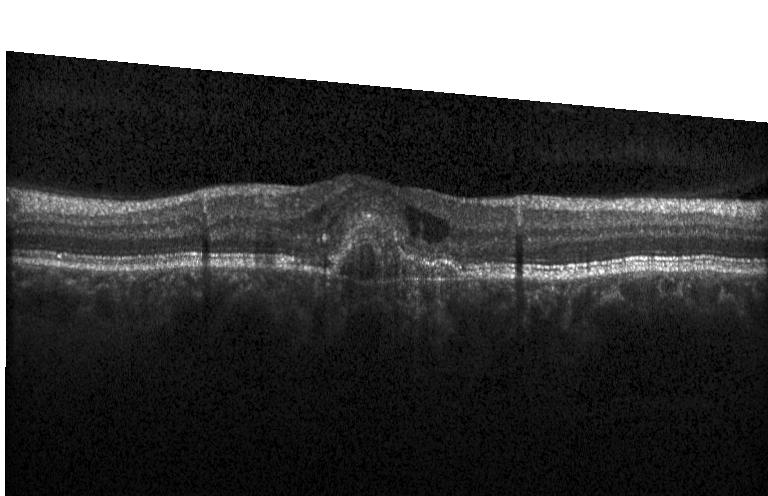 Assessment: a choroidal neovascular membrane.